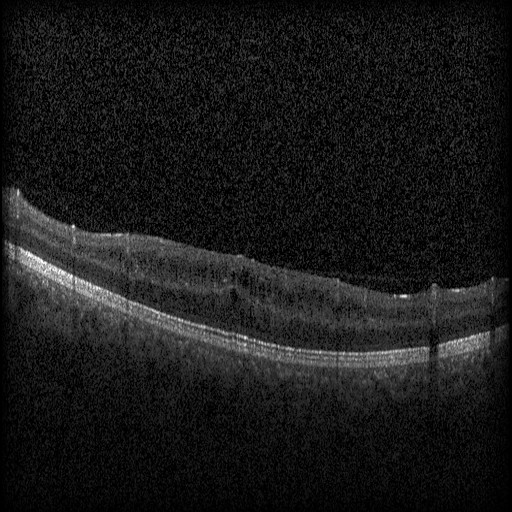
OCT B-scan. Acquired on a Heidelberg Spectralis
Impression: diabetic macular edema (DME).